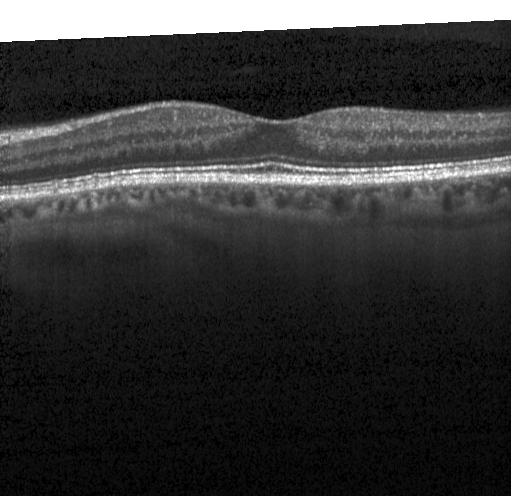

Optical coherence tomography B-scan.
This B-scan demonstrates no CNV, DME, or drusen.